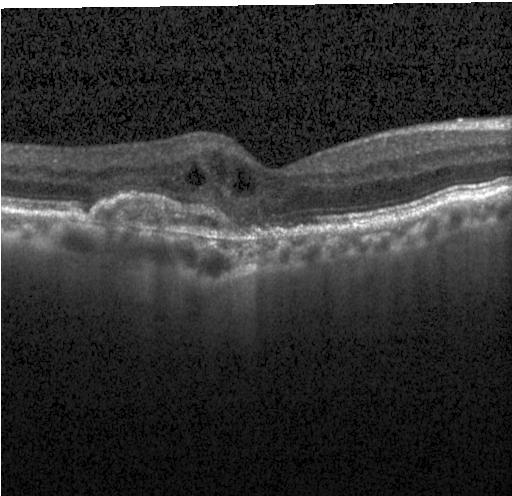
Diagnosis: a choroidal neovascular membrane.